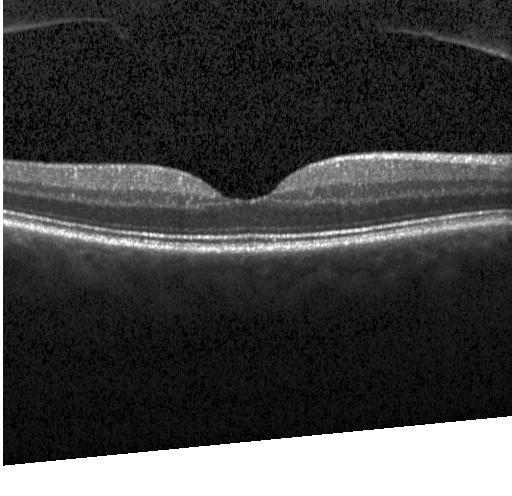
Neither choroidal neovascularization, diabetic macular edema, nor drusen.